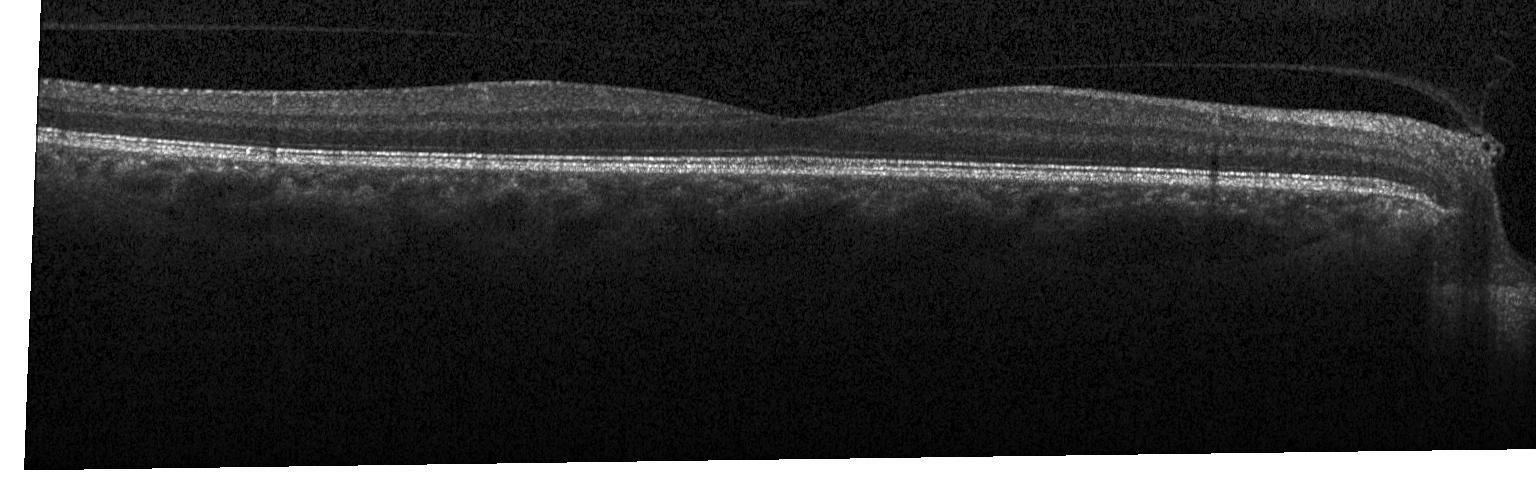

Horizontal scan through the fovea, OCT B-scan, spectral-domain OCT, Heidelberg Spectralis OCT system — OCT finding: no choroidal neovascularization, no diabetic macular edema, and no drusen.